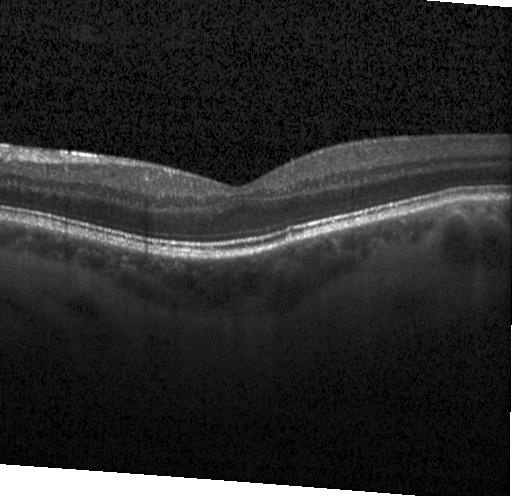 OCT line scan — Diagnosis: no CNV, no DME, and no drusen.